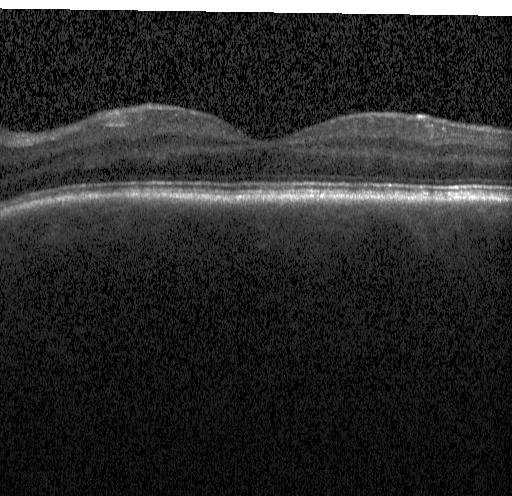 OCT B-scan — Diagnosis: no evidence of choroidal neovascularization, diabetic macular edema, or drusen.